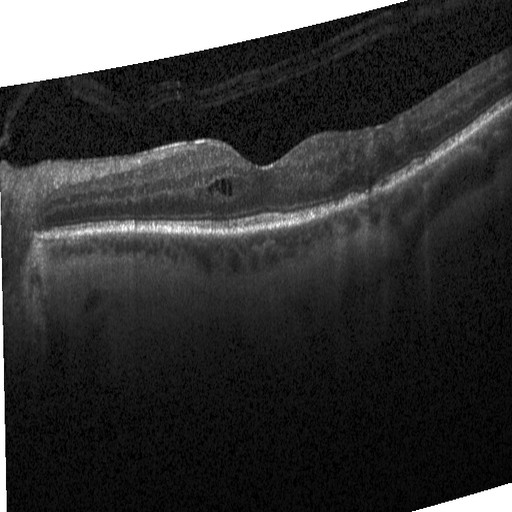
Horizontal scan through the fovea; spectral-domain optical coherence tomography; acquired on a Heidelberg Spectralis; OCT line scan — Finding: DME.